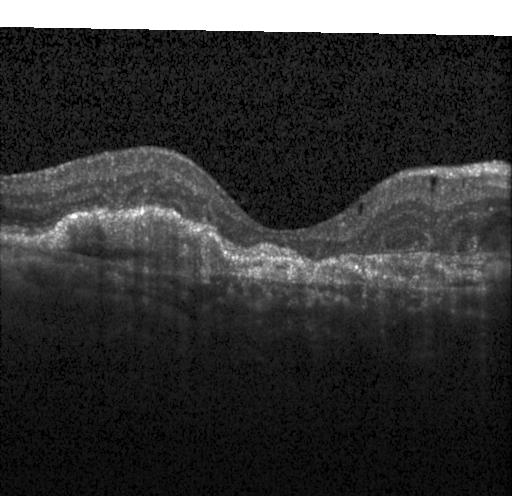
Macular OCT: CNV.